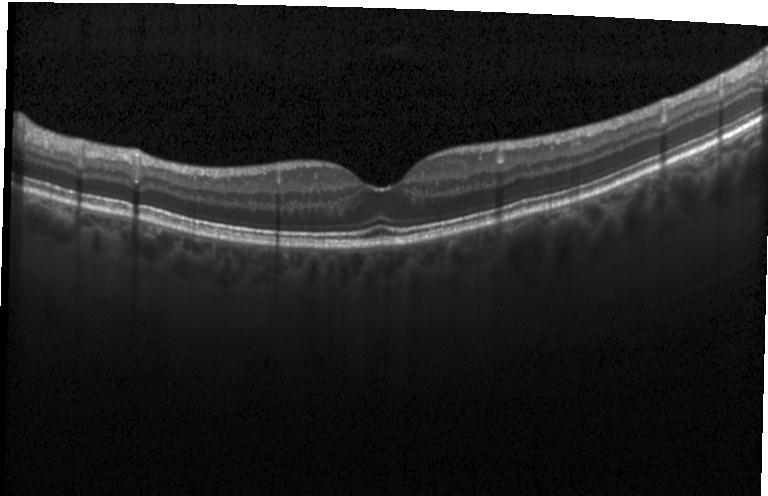 Diagnosis: neither choroidal neovascularization, diabetic macular edema, nor drusen.